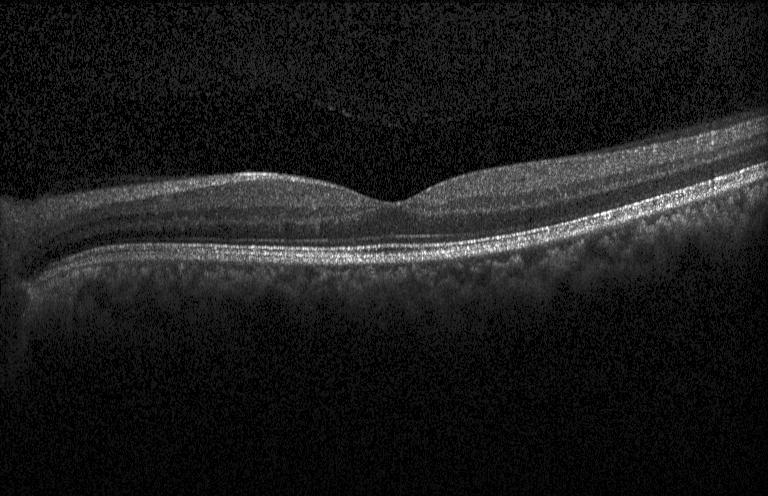

Finding: no evidence of CNV, DME, or drusen.